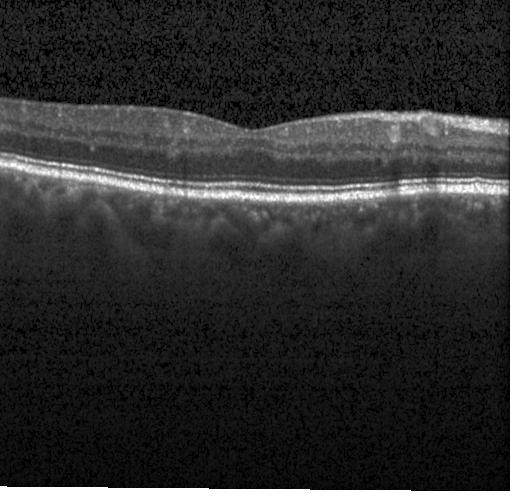

Spectral-domain OCT B-scan: no choroidal neovascularization, diabetic macular edema, or drusen.